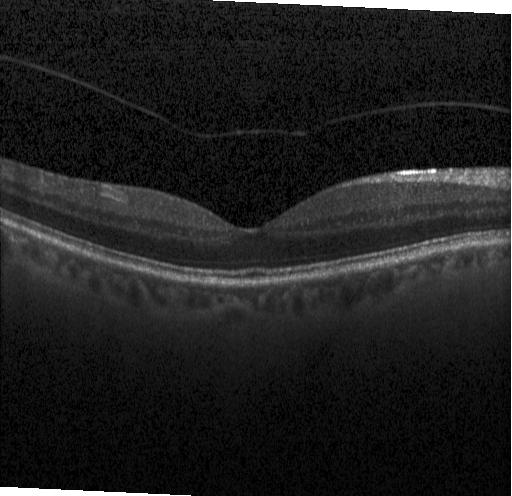
Optical coherence tomography B-scan · Heidelberg Spectralis OCT system · spectral-domain optical coherence tomography. Diagnosis: no evidence of choroidal neovascularization, diabetic macular edema, or drusen.